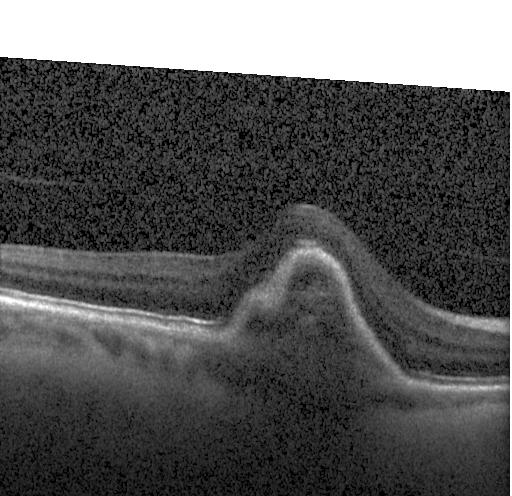

OCT B-scan. Instrument: Heidelberg Spectralis. Spectral-domain OCT — Dx: choroidal neovascularization (CNV).